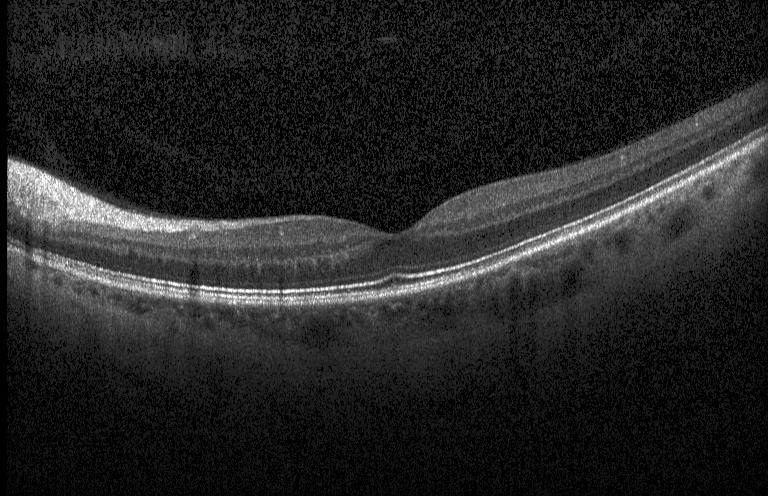

OCT line scan, macular scan
Diagnosis: no choroidal neovascularization, no diabetic macular edema, and no drusen.